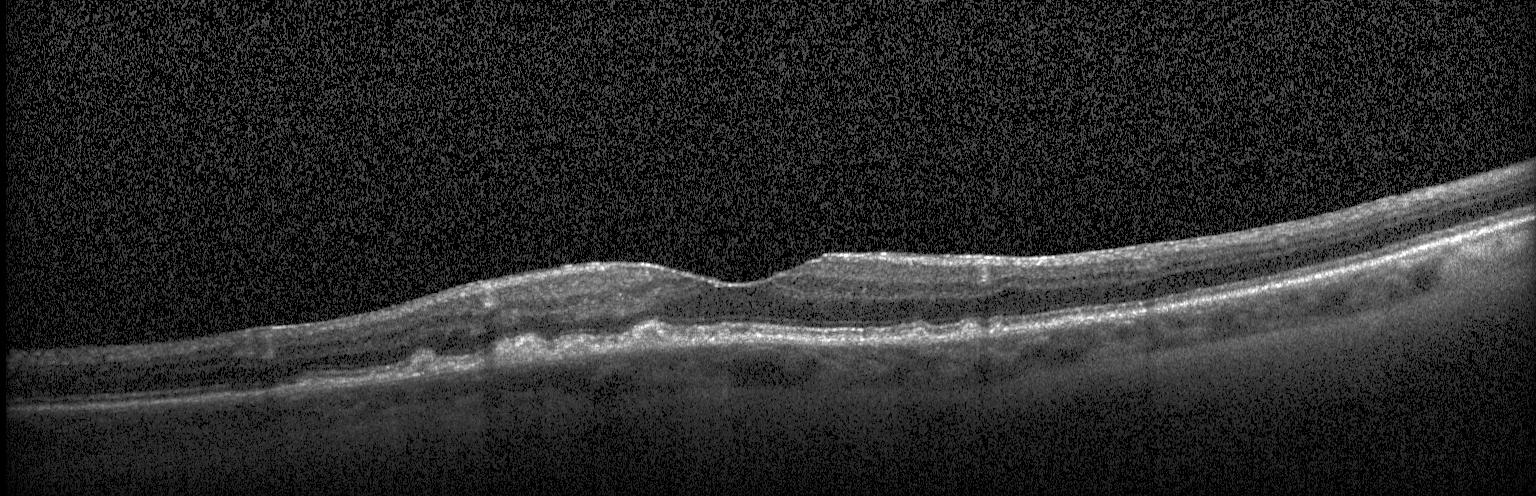
Dx: sub-RPE drusenoid deposits.